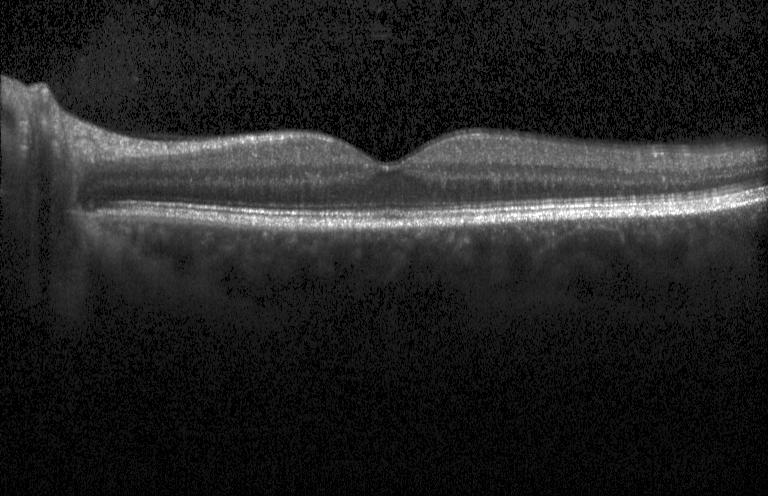

Retinal OCT B-scan
The scan shows no choroidal neovascularization, no diabetic macular edema, and no drusen.